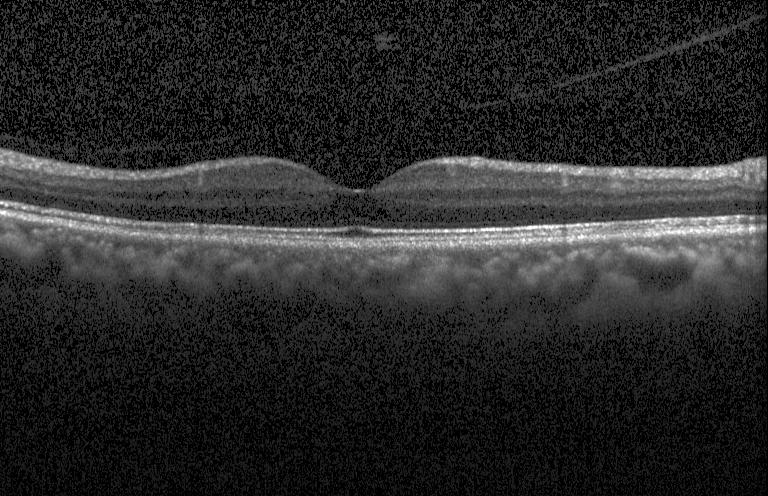 Impression: no choroidal neovascularization, diabetic macular edema, or drusen.